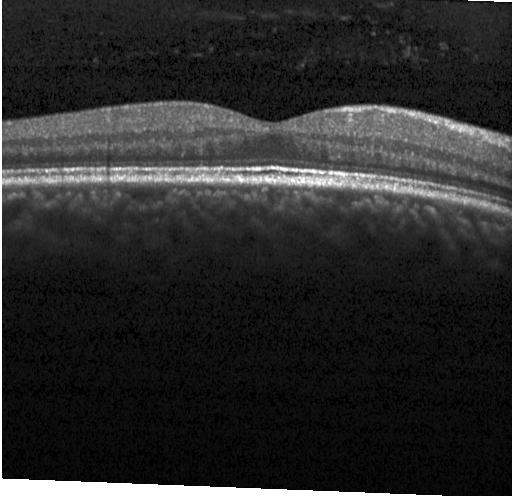
SD-OCT. Optical coherence tomography scan. Diagnosis: no choroidal neovascularization, no diabetic macular edema, and no drusen.